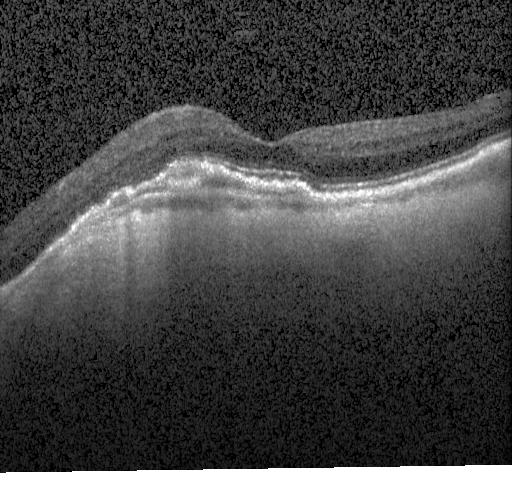

Macular OCT demonstrating choroidal neovascularization.